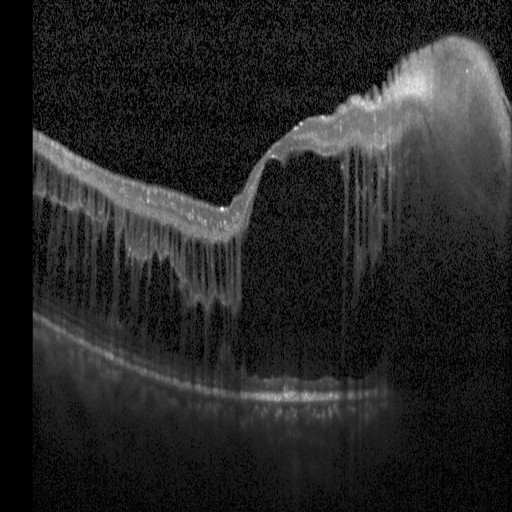

Retinal OCT cross-section.
Impression: diabetic macular edema (DME).